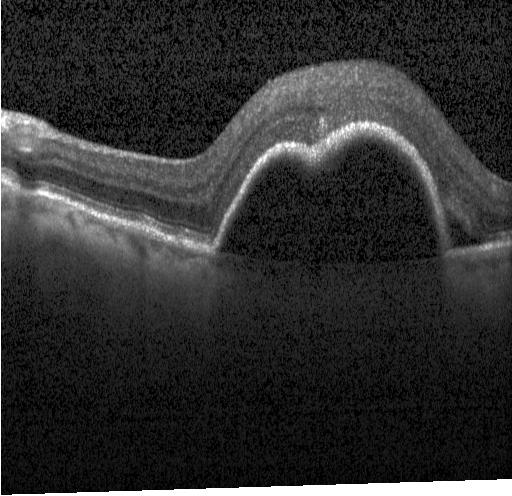

Finding: a choroidal neovascular membrane.